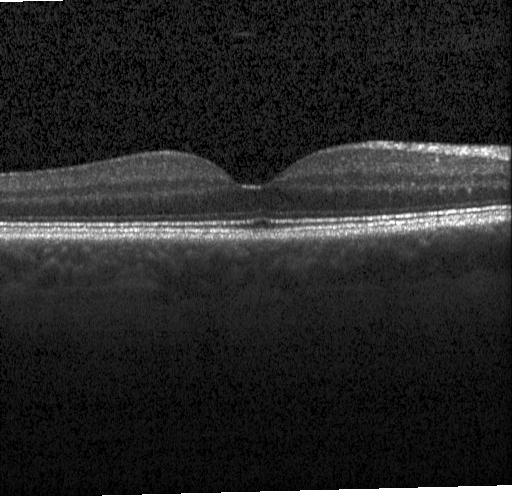 Diagnosis: no choroidal neovascularization, no diabetic macular edema, and no drusen.